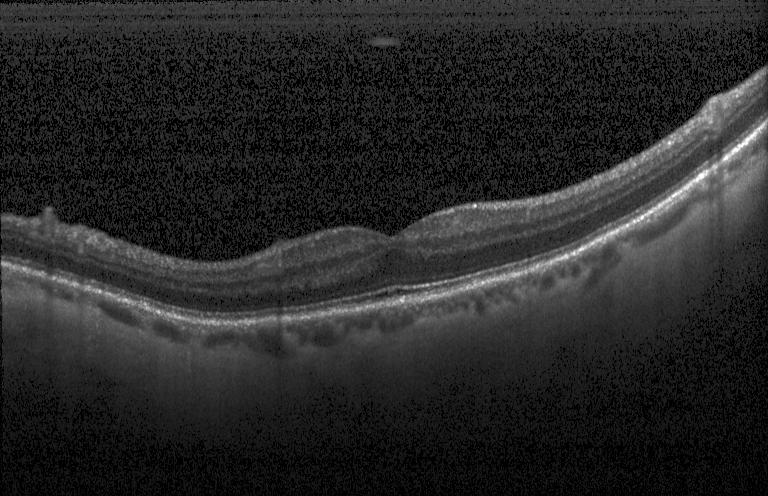 OCT B-scan showing neither choroidal neovascularization, diabetic macular edema, nor drusen.